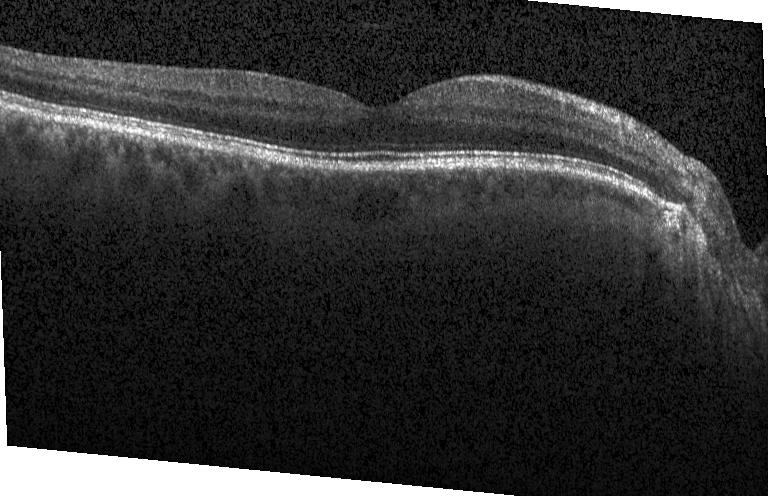 Neither CNV, DME, nor drusen.